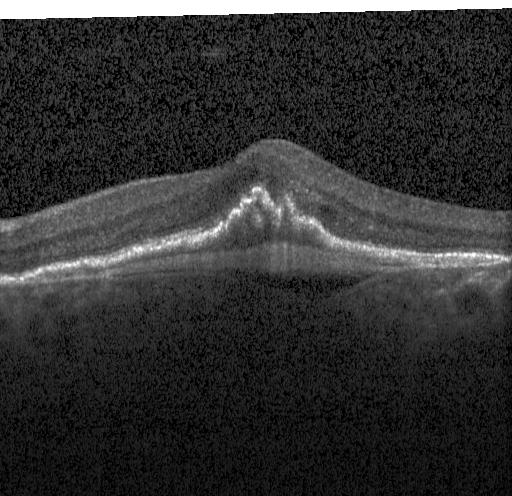

Optical coherence tomography B-scan · through the macula
Impression: a choroidal neovascular membrane.